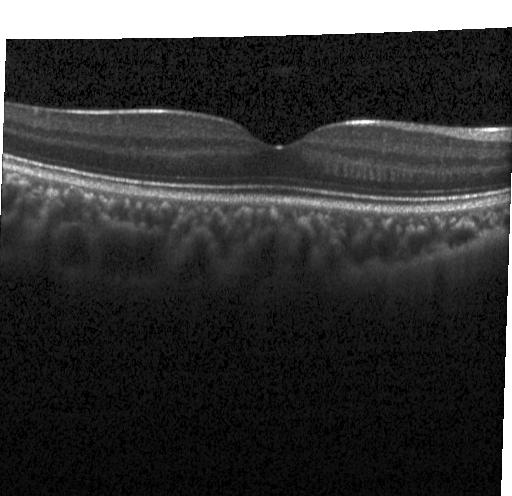

Acquired on a Heidelberg Spectralis; optical coherence tomography B-scan; through the macula; spectral-domain OCT — Assessment: no CNV, DME, or drusen.